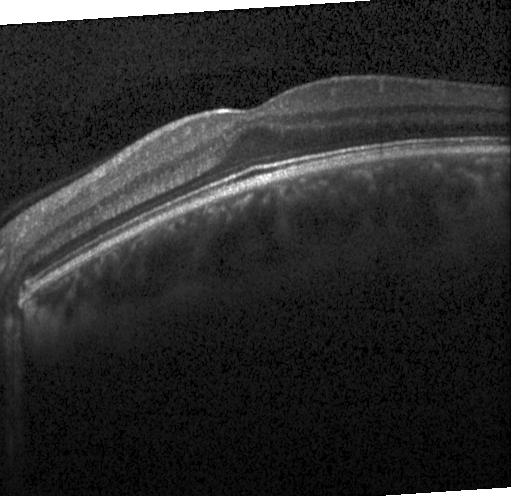 Diagnosis: no evidence of choroidal neovascularization, diabetic macular edema, or drusen.